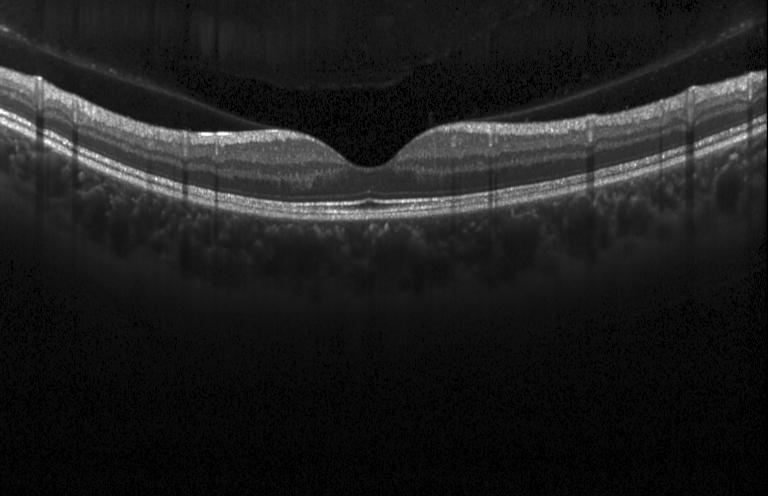 OCT scan showing no choroidal neovascularization, no diabetic macular edema, and no drusen.